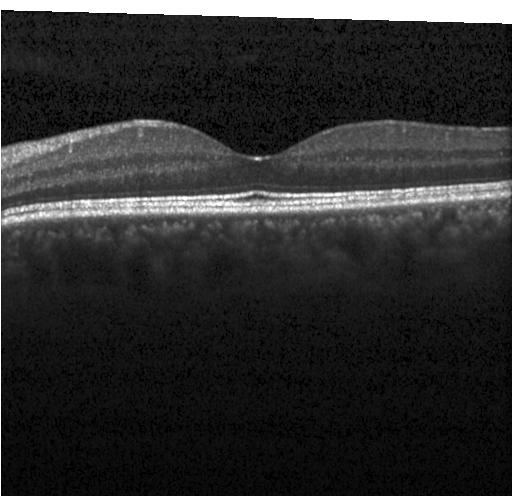

Diagnosis: no choroidal neovascularization, no diabetic macular edema, and no drusen.